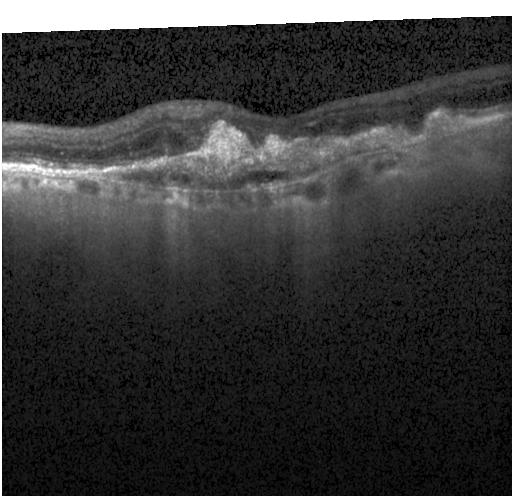 Diagnosis: a choroidal neovascular membrane.